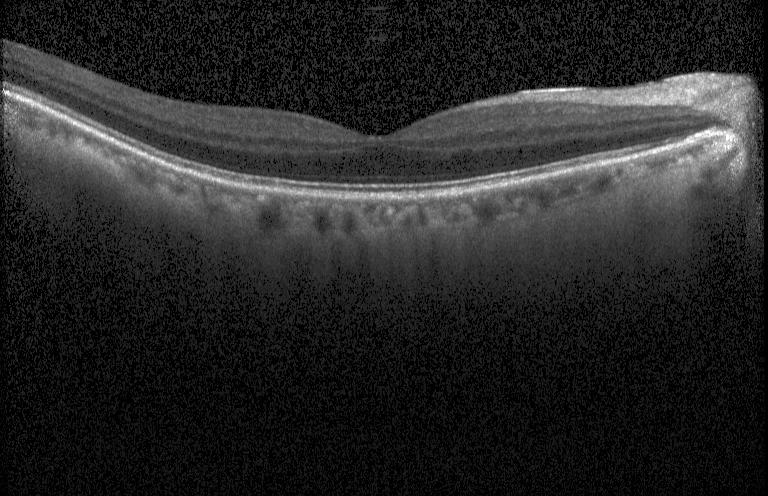
OCT finding: no evidence of choroidal neovascularization, diabetic macular edema, or drusen.